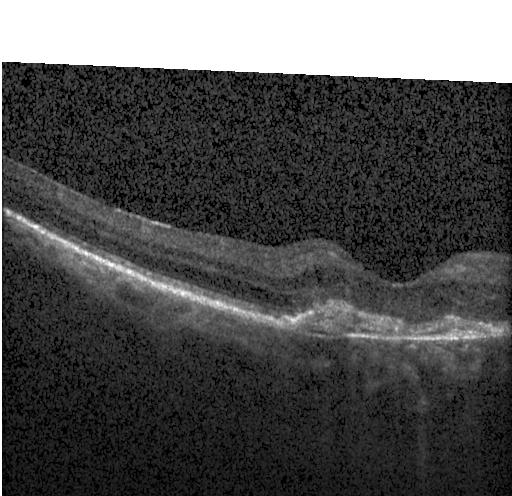 OCT B-scan — The scan shows a choroidal neovascular membrane.